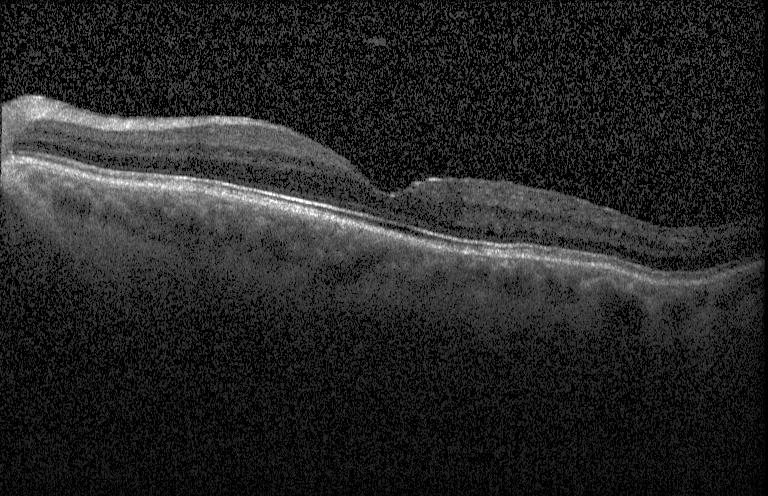

Macular scan; spectral-domain optical coherence tomography; instrument: Heidelberg Spectralis; retinal OCT B-scan. No evidence of choroidal neovascularization, diabetic macular edema, or drusen.